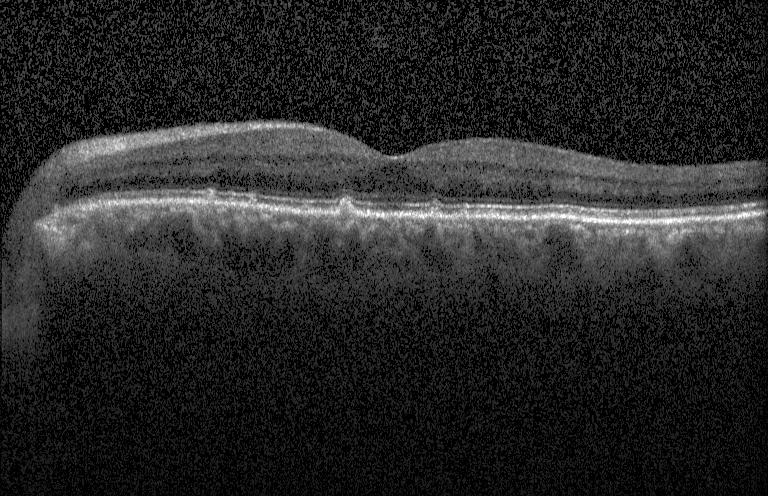

Assessment: drusen.